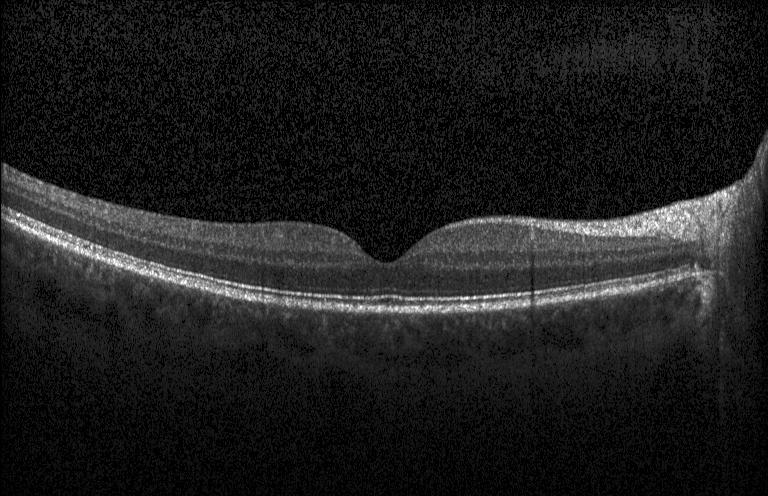

Optical coherence tomography scan · acquired on a Heidelberg Spectralis · fovea-centered · spectral-domain optical coherence tomography.
Dx: no choroidal neovascularization, no diabetic macular edema, and no drusen.